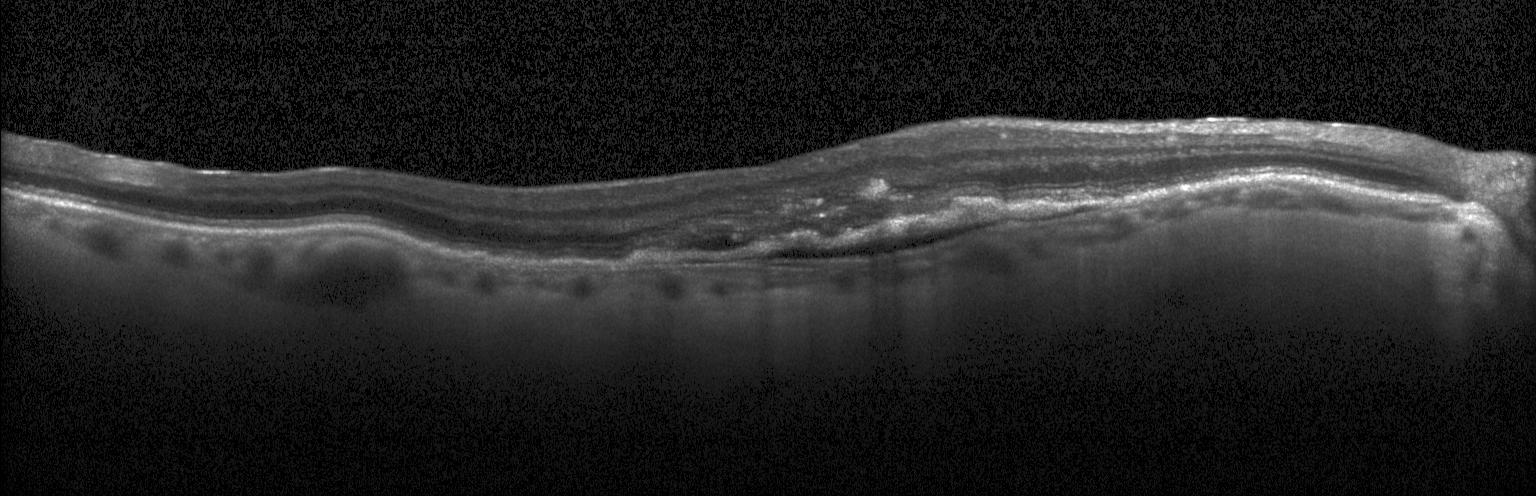

Impression: choroidal neovascularization.